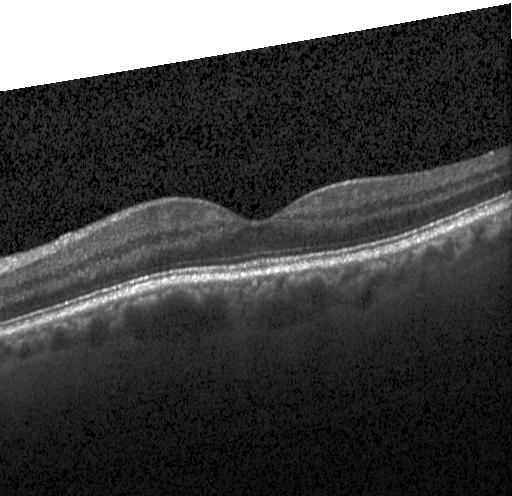
Acquired on a Heidelberg Spectralis · retinal OCT B-scan.
This B-scan demonstrates no evidence of CNV, DME, or drusen.